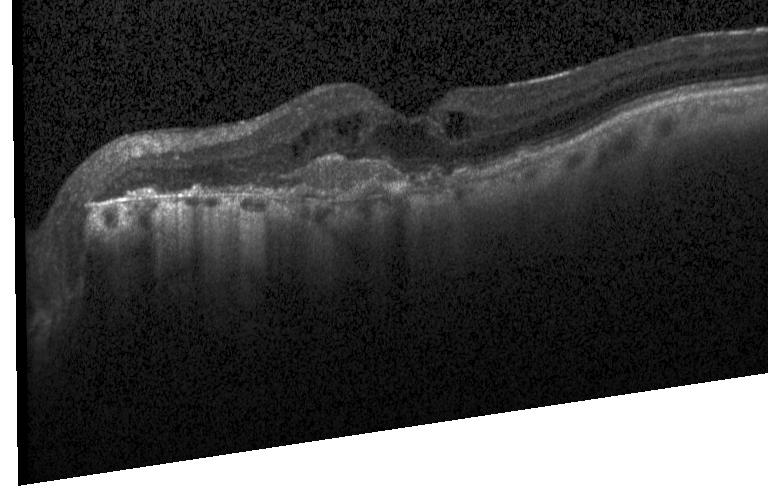 Diagnosis: a choroidal neovascular membrane.